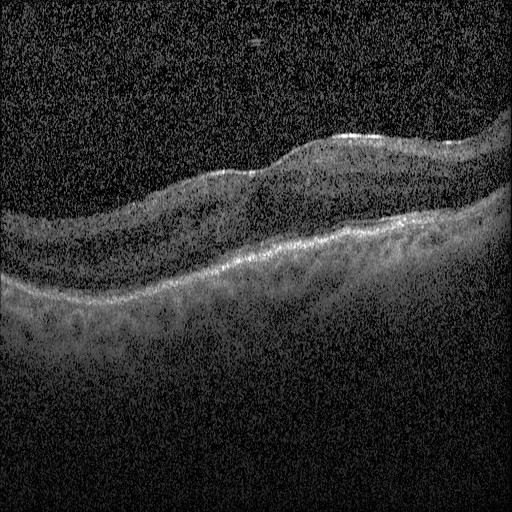 DME.